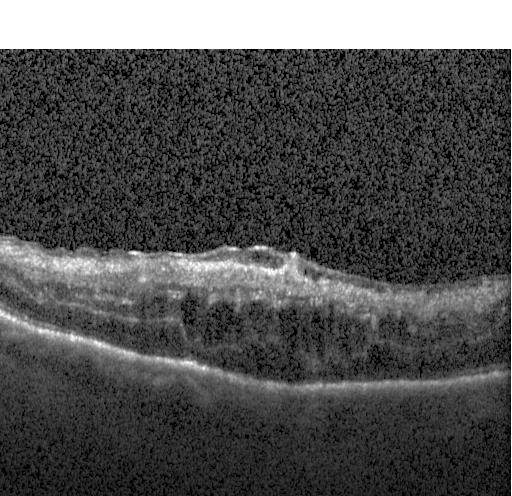
Spectral-domain OCT B-scan: DME.